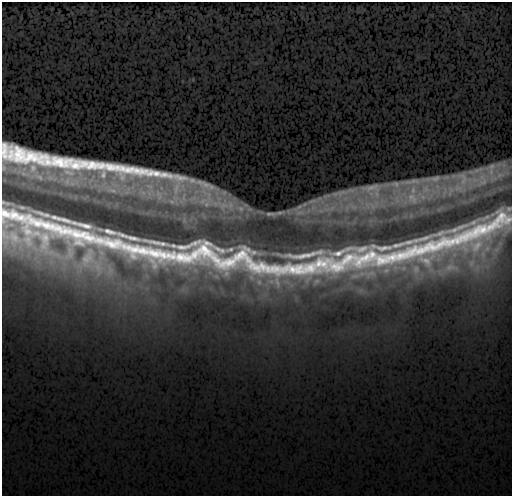 Instrument: Heidelberg Spectralis · spectral-domain OCT · OCT B-scan.
Diagnosis: drusen.